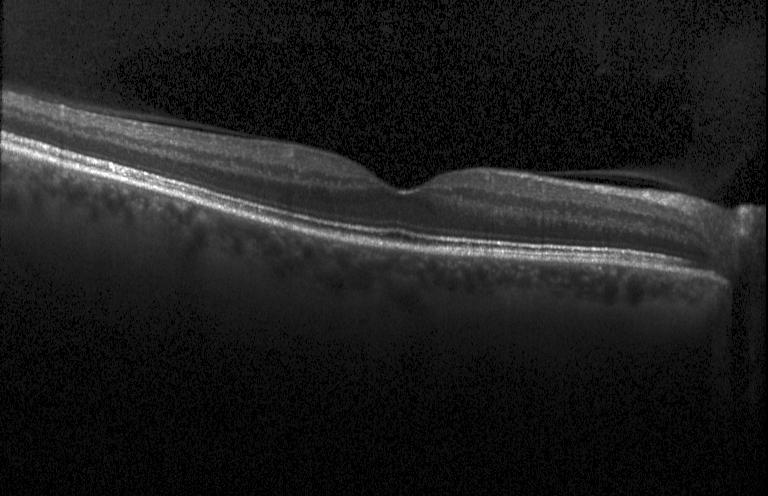
Retinal OCT cross-section. Finding: neither CNV, DME, nor drusen.